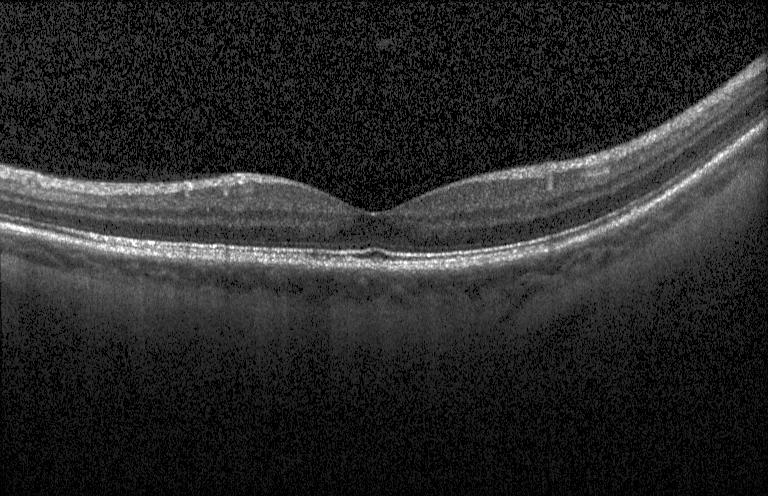

OCT line scan. Diagnosis: neither CNV, DME, nor drusen.